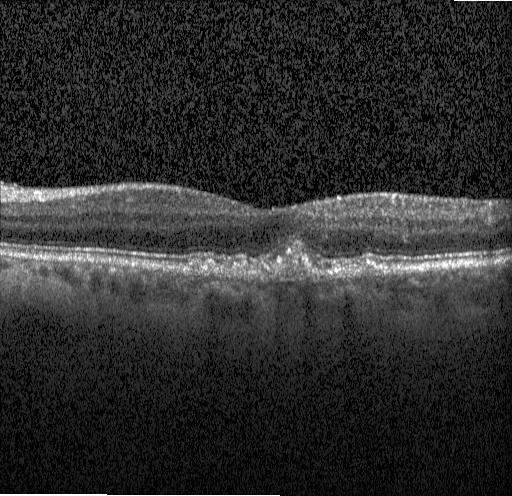
OCT B-scan.
Diagnosis: sub-RPE drusenoid deposits.